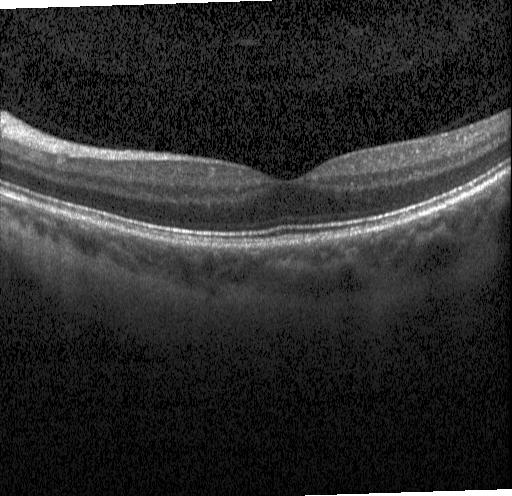

Diagnosis: no choroidal neovascularization, no diabetic macular edema, and no drusen.